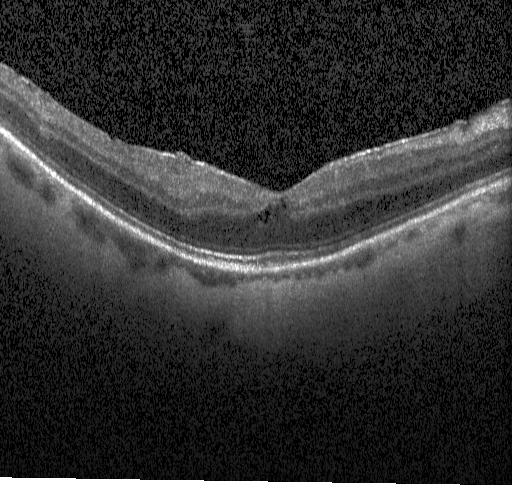
Spectral-domain OCT; horizontal scan through the fovea; retinal OCT B-scan; Heidelberg Spectralis — Diagnosis: DME.